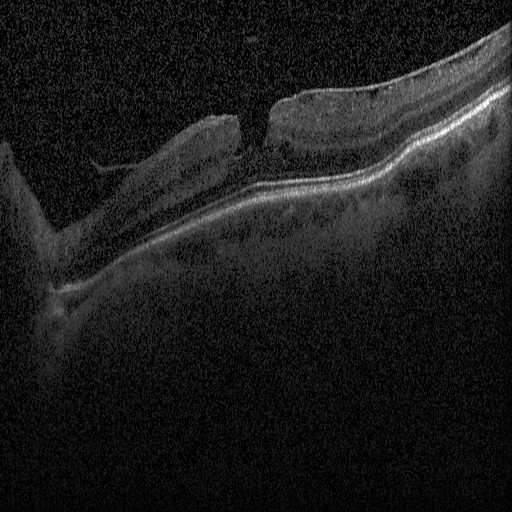
Impression: DME.